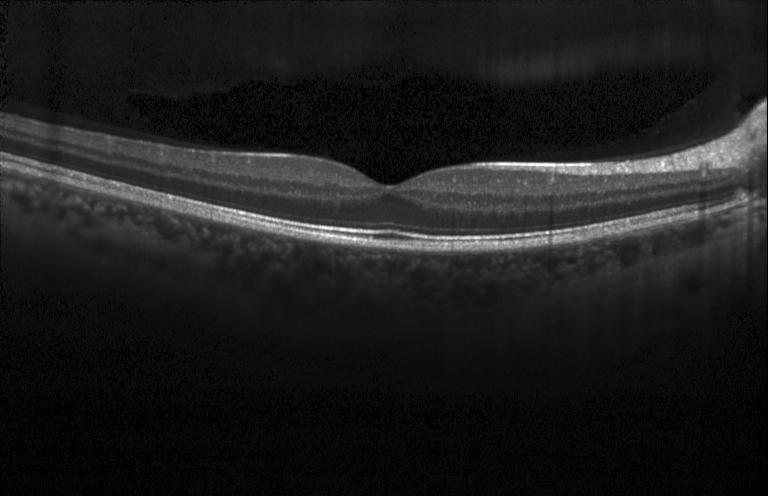

Spectral-domain OCT; OCT line scan; centered on the fovea.
Diagnosis: neither choroidal neovascularization, diabetic macular edema, nor drusen.